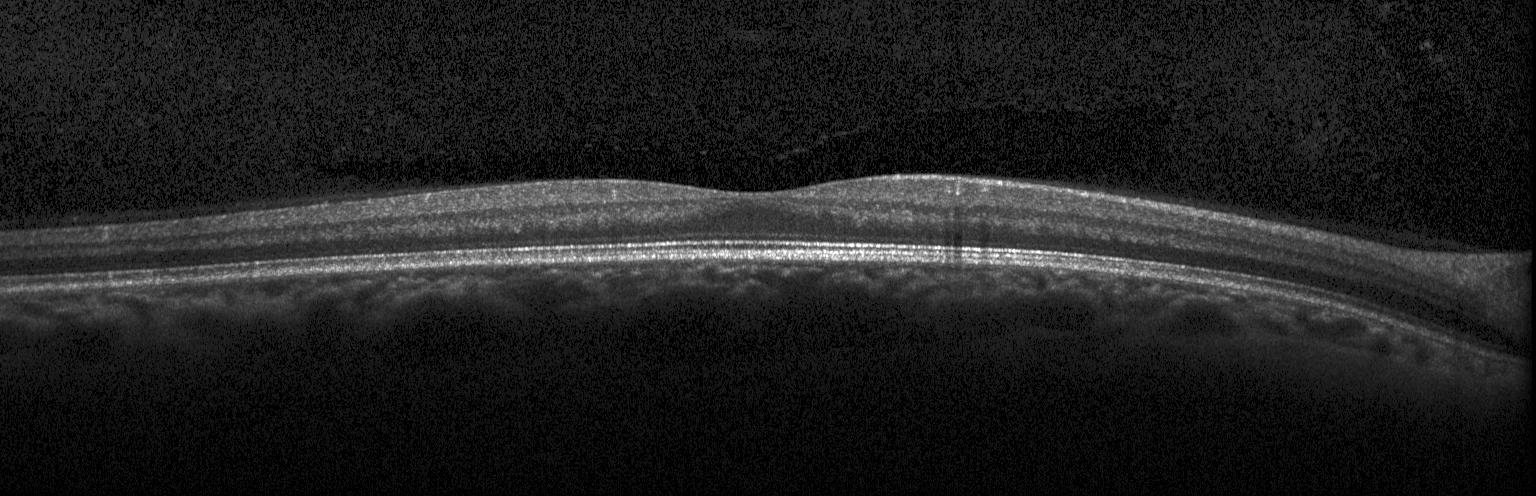

Retinal OCT B-scan — OCT finding: no choroidal neovascularization, diabetic macular edema, or drusen.